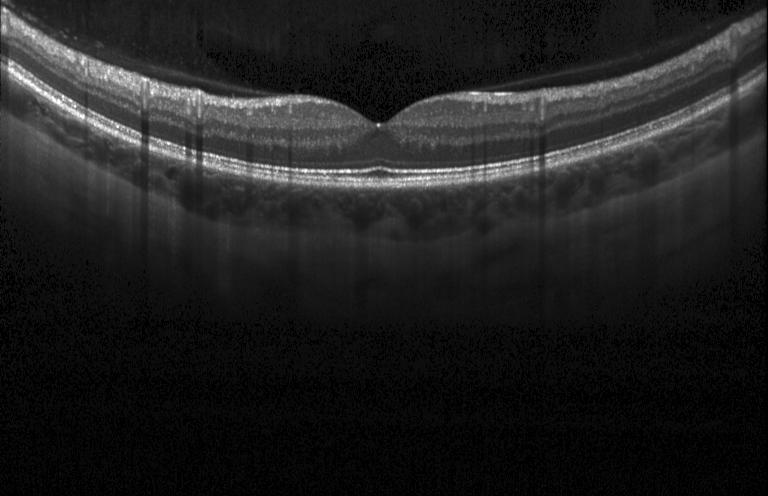 Assessment: no choroidal neovascularization, diabetic macular edema, or drusen.